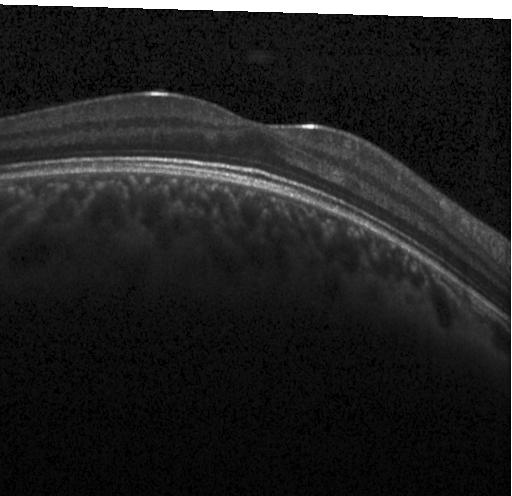 OCT B-scan showing no choroidal neovascularization, no diabetic macular edema, and no drusen.